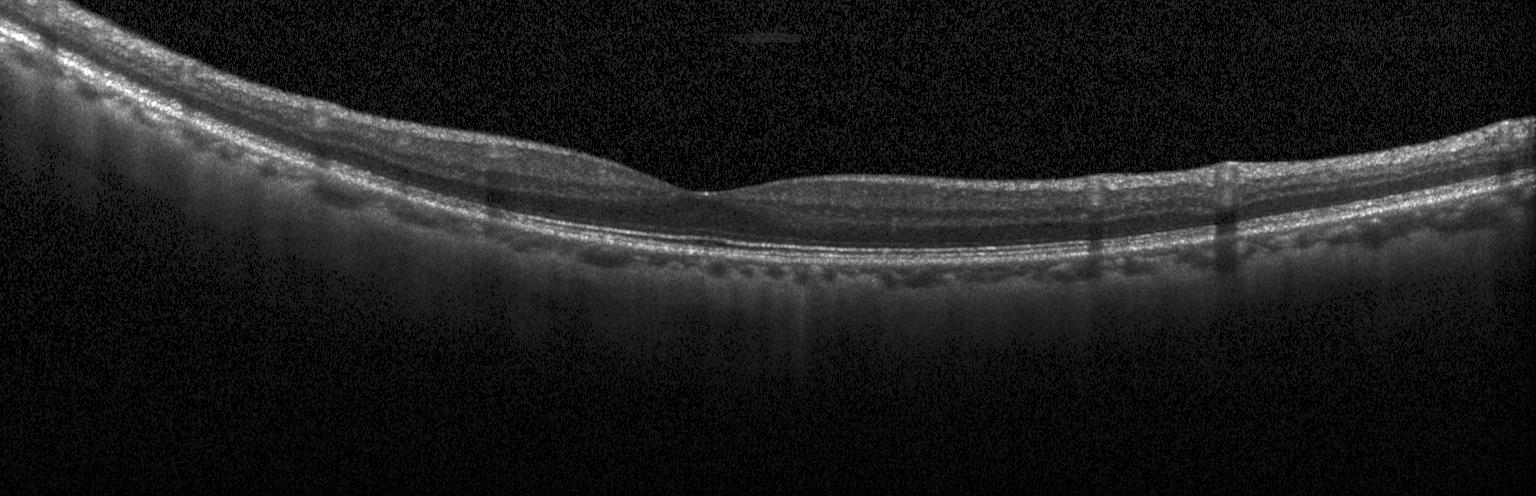
Optical coherence tomography scan — Diagnosis: no choroidal neovascularization, no diabetic macular edema, and no drusen.